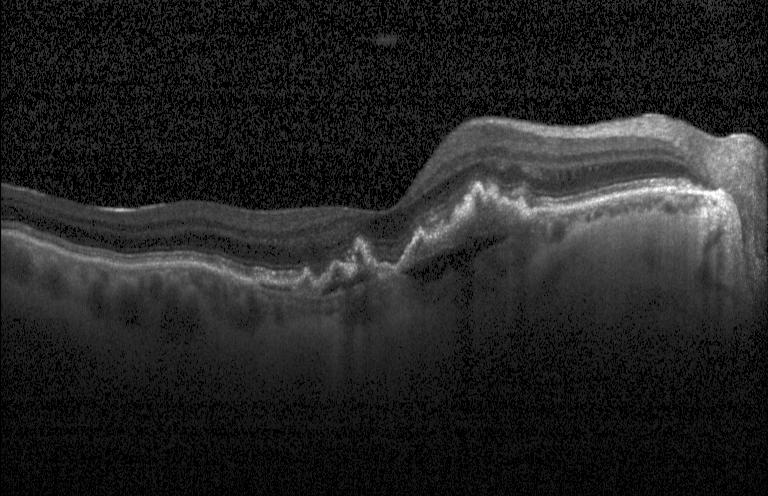 Acquired on a Heidelberg Spectralis · OCT B-scan
A choroidal neovascular membrane.